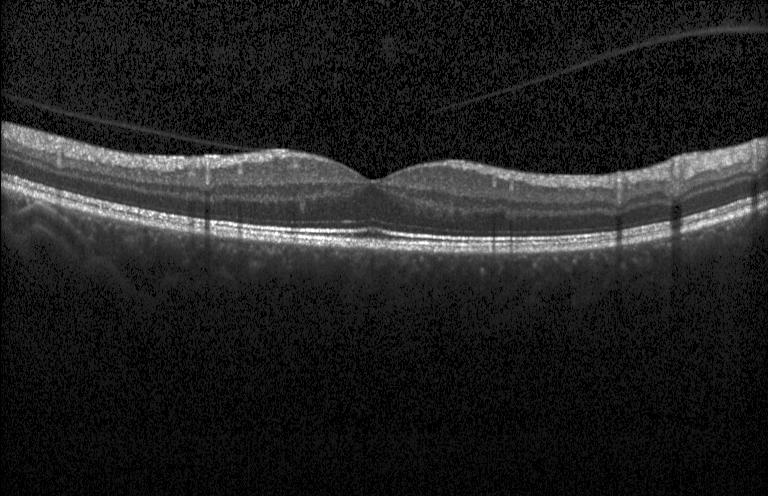
OCT scan showing no CNV, no DME, and no drusen.